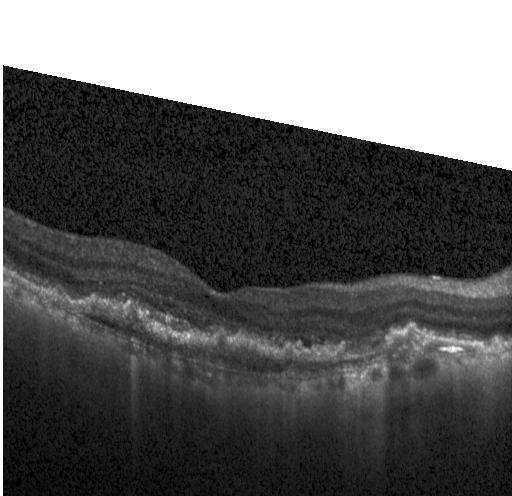

Heidelberg Spectralis OCT system, retinal OCT B-scan, spectral-domain optical coherence tomography, macular scan. Choroidal neovascularization.